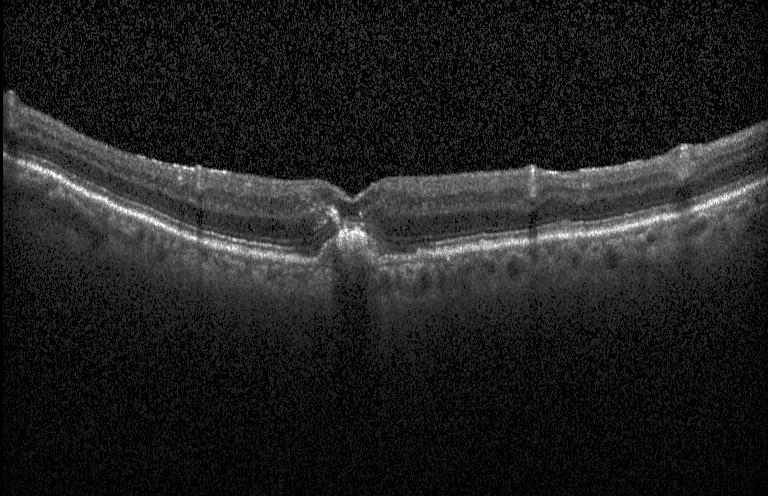 Retinal OCT cross-section · SD-OCT · fovea-centered.
Finding: CNV.